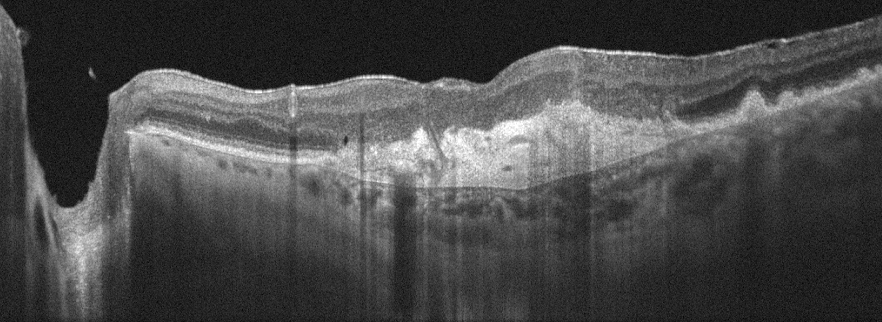
Left eye, Optovue Avanti RTVue XR, optical coherence tomography scan
Age-related macular degeneration.